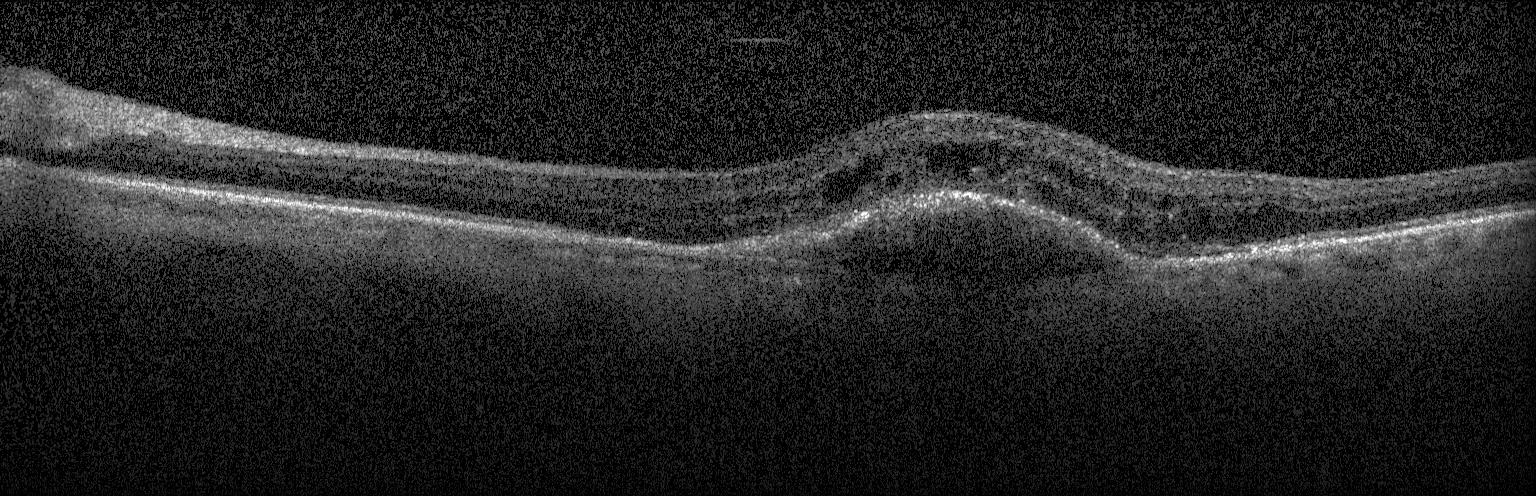
OCT B-scan. Instrument: Heidelberg Spectralis. Fovea-centered.
Macular OCT: a choroidal neovascular membrane.